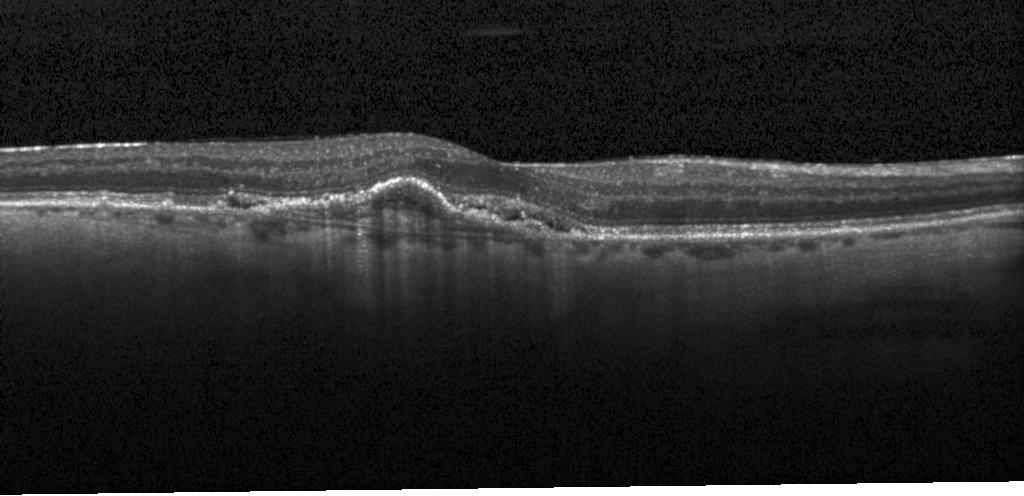
Macular OCT demonstrating a choroidal neovascular membrane.